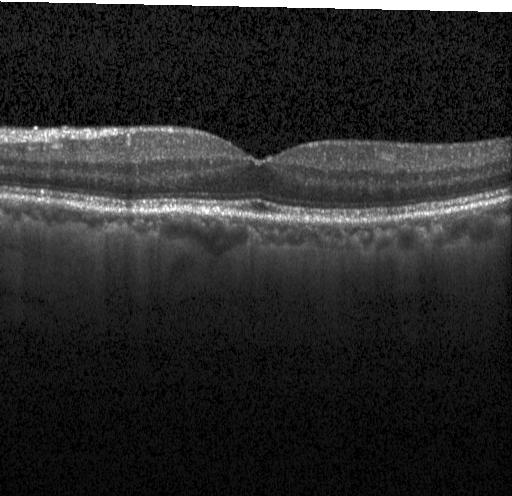

Optical coherence tomography scan — Assessment: neither CNV, DME, nor drusen.